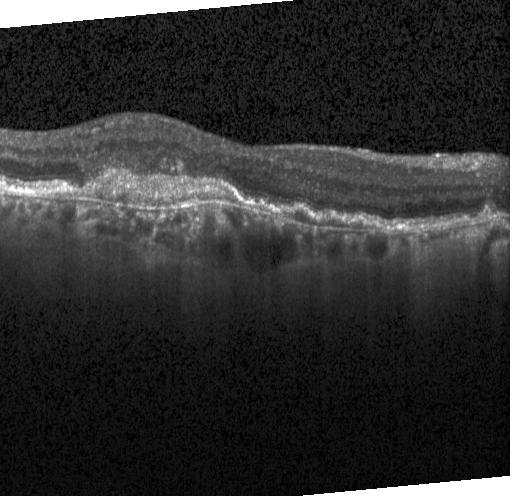 A choroidal neovascular membrane.